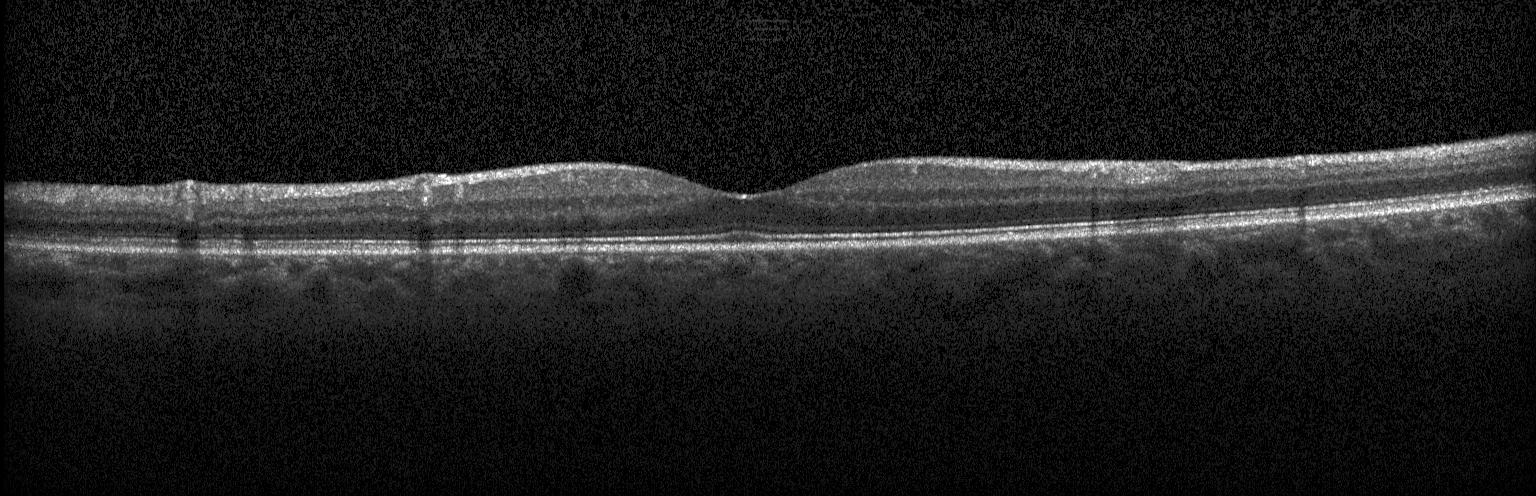
Macular OCT: no CNV, DME, or drusen.